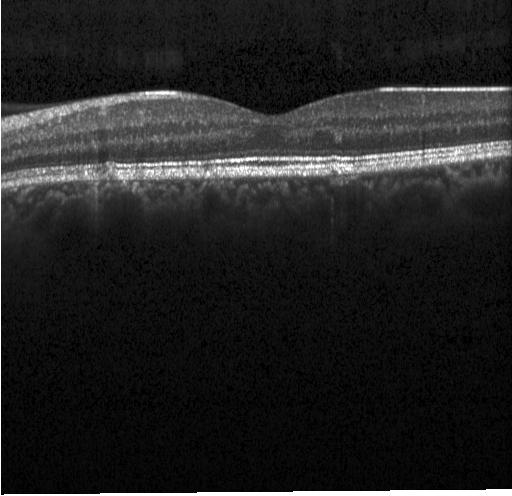
OCT scan showing no evidence of CNV, DME, or drusen.